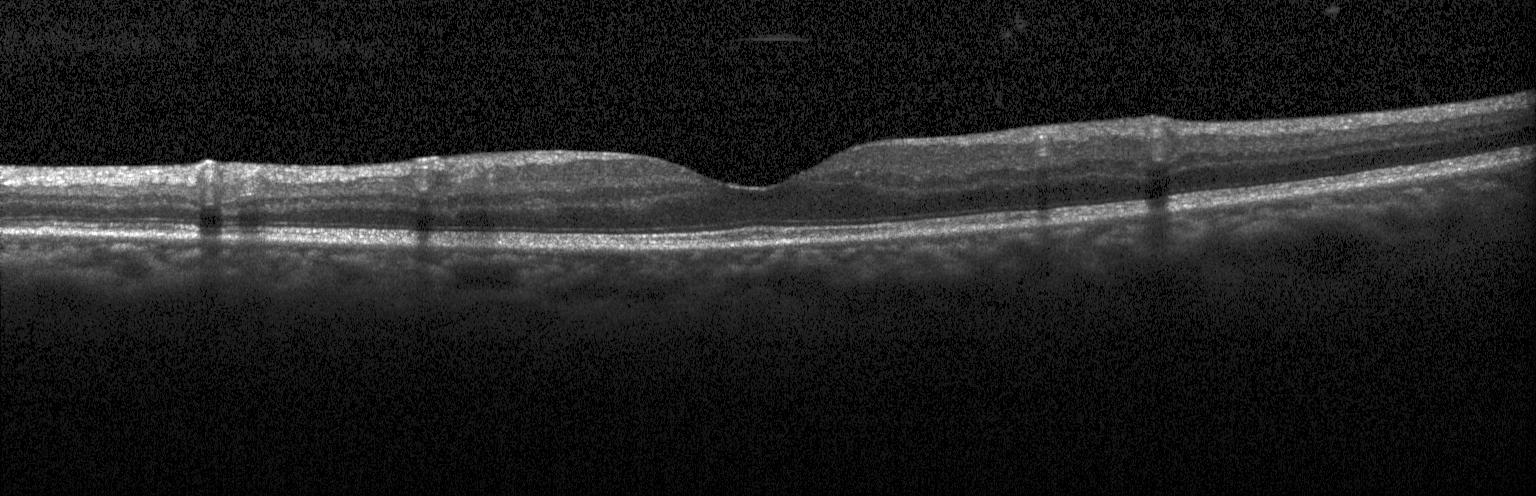

Impression: no CNV, no DME, and no drusen.